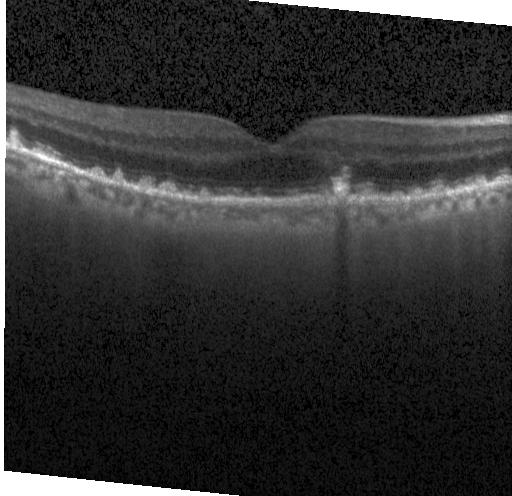

OCT line scan — Finding: drusen.